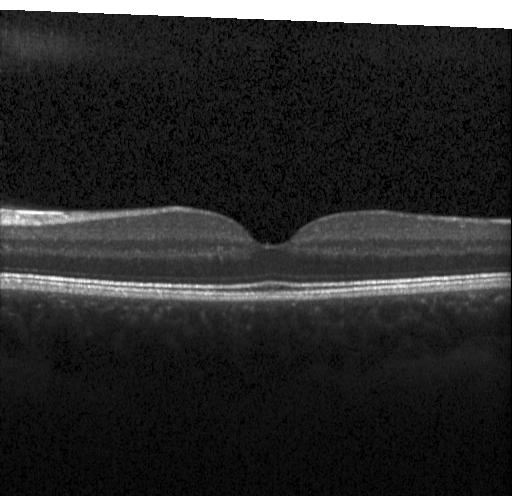 OCT B-scan showing no choroidal neovascularization, diabetic macular edema, or drusen.